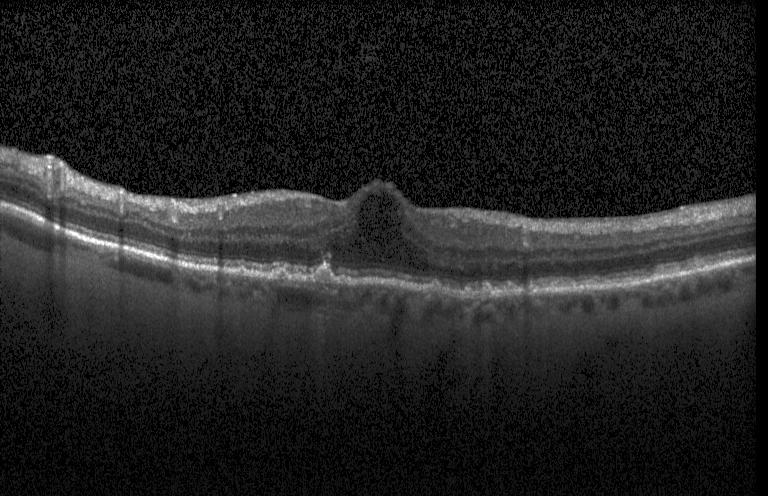 OCT scan showing choroidal neovascularization.